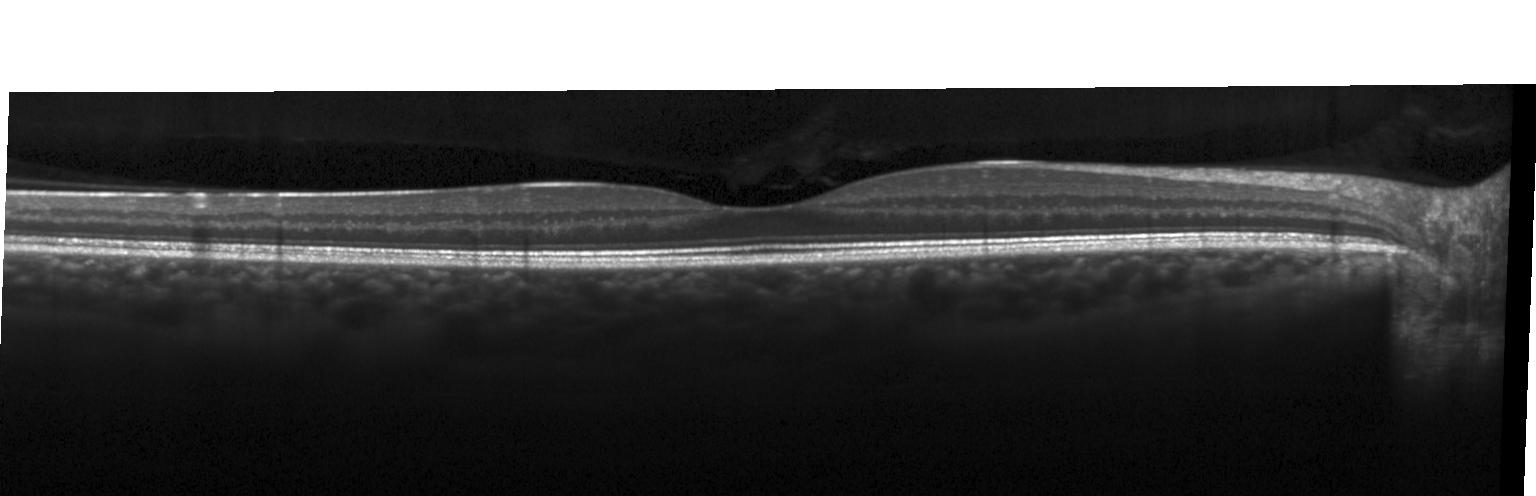 SD-OCT; optical coherence tomography scan — Diagnosis: no choroidal neovascularization, diabetic macular edema, or drusen.